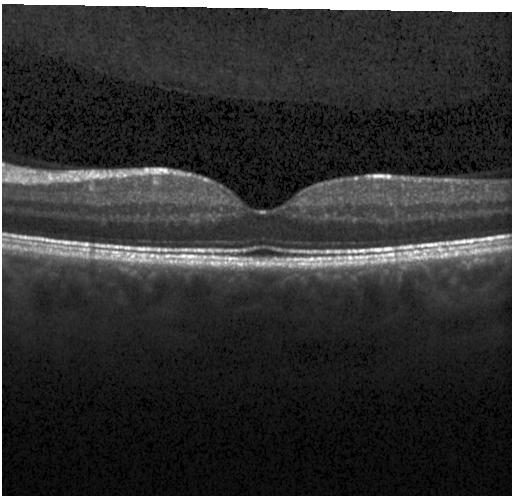 The scan shows neither choroidal neovascularization, diabetic macular edema, nor drusen.